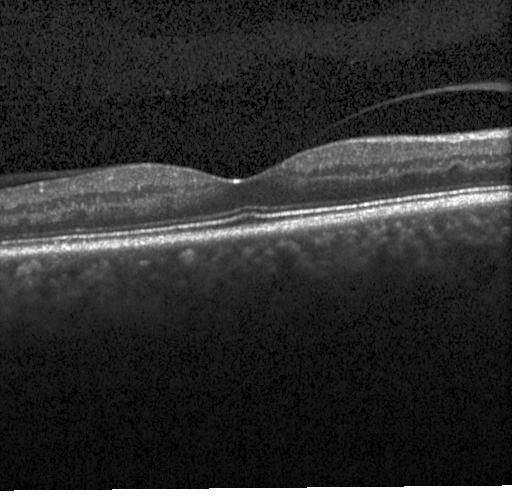 Optical coherence tomography B-scan. Macular OCT: no evidence of CNV, DME, or drusen.